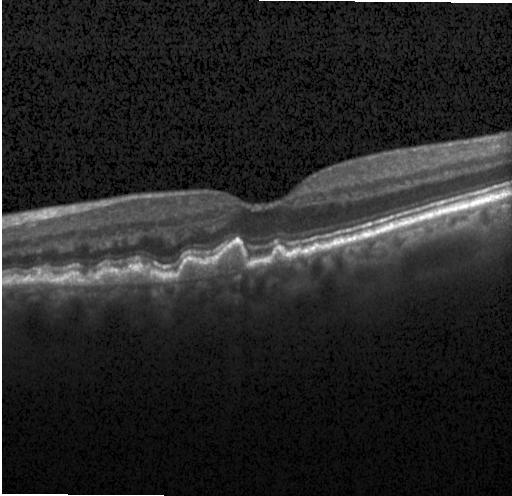 The scan shows drusen.